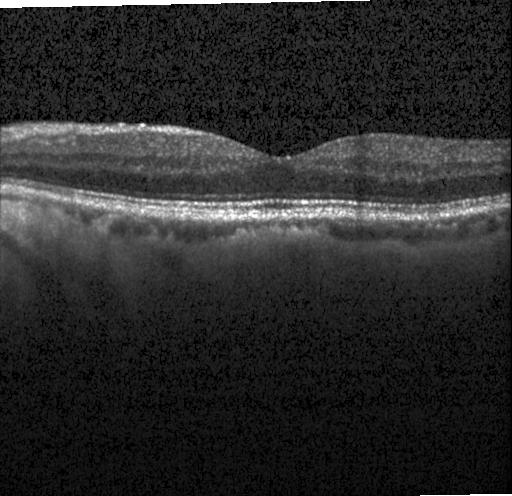 Acquired on a Heidelberg Spectralis, optical coherence tomography scan, spectral-domain optical coherence tomography, centered on the fovea — This B-scan demonstrates no CNV, DME, or drusen.